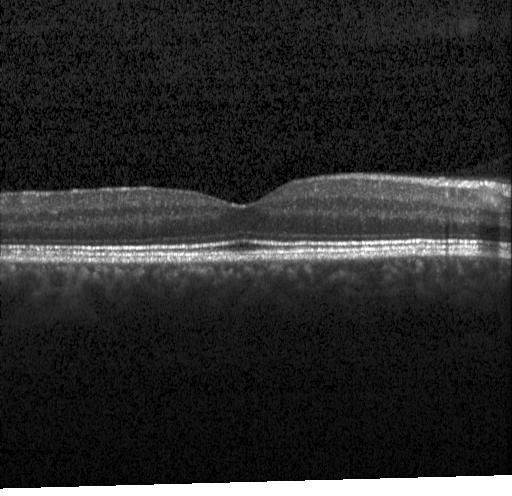
Optical coherence tomography scan. Spectral-domain OCT. Heidelberg Spectralis OCT system.
Dx: no choroidal neovascularization, no diabetic macular edema, and no drusen.